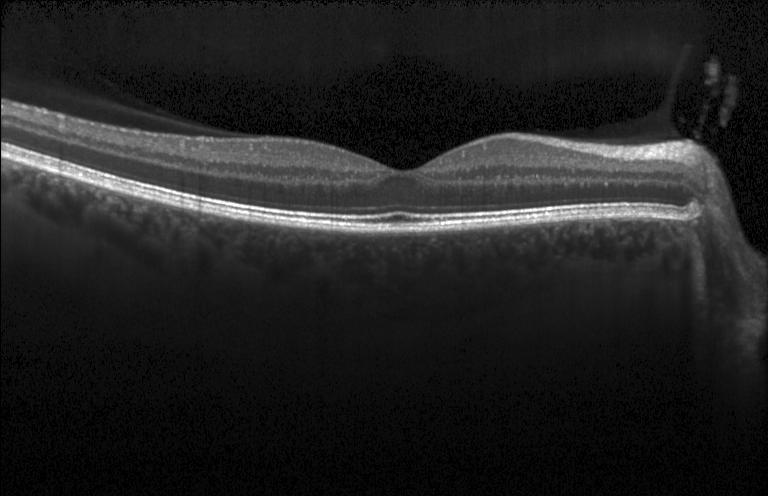
OCT B-scan, spectral-domain OCT
The scan shows neither choroidal neovascularization, diabetic macular edema, nor drusen.